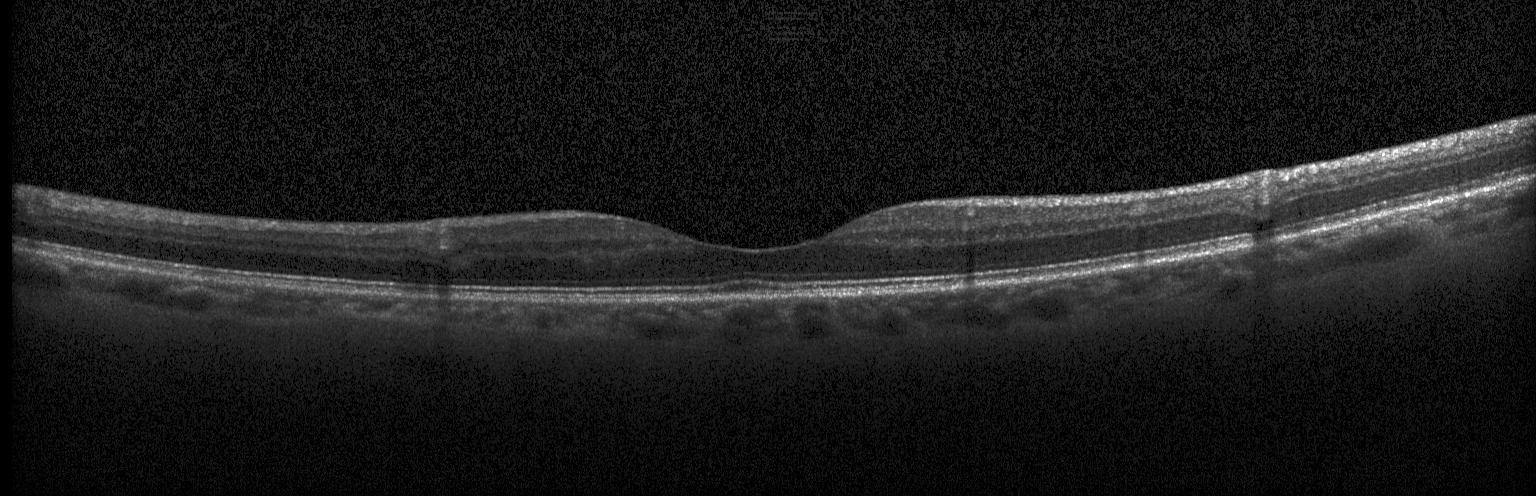
Acquired on a Heidelberg Spectralis. Optical coherence tomography scan
Diagnosis: no choroidal neovascularization, diabetic macular edema, or drusen.